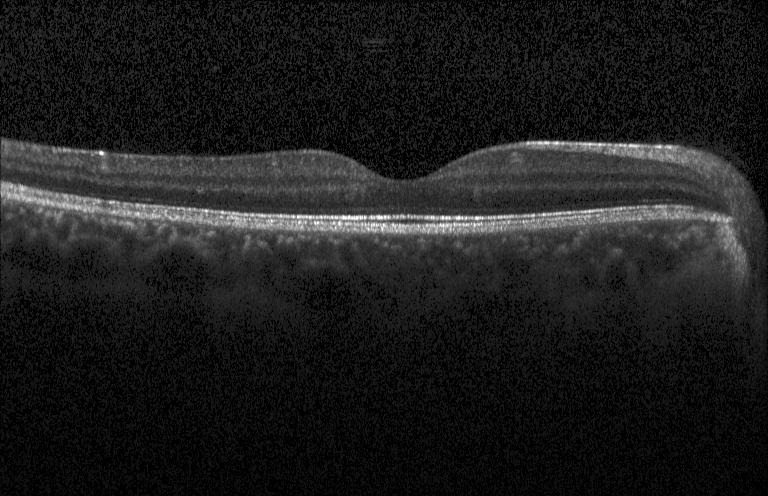 Impression: neither CNV, DME, nor drusen.